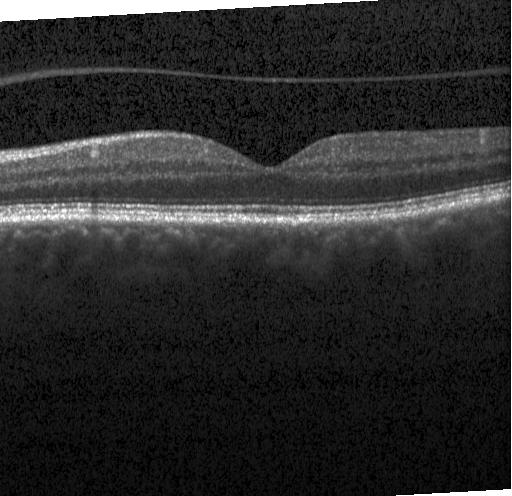

Macular scan. Spectral-domain optical coherence tomography. Heidelberg Spectralis. OCT line scan — Diagnosis: neither choroidal neovascularization, diabetic macular edema, nor drusen.